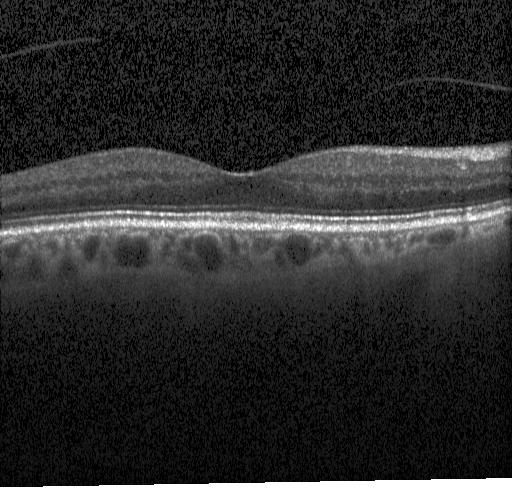
Spectral-domain OCT. Heidelberg Spectralis OCT system. Retinal OCT B-scan. Centered on the fovea
Finding: no choroidal neovascularization, no diabetic macular edema, and no drusen.